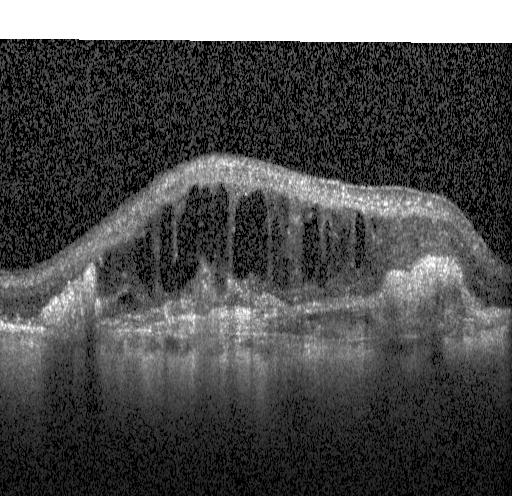 Impression: a choroidal neovascular membrane.